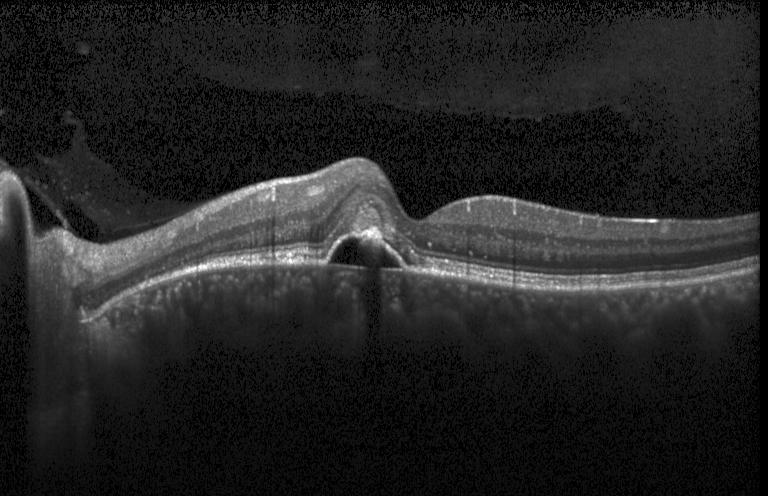

Finding: a choroidal neovascular membrane.